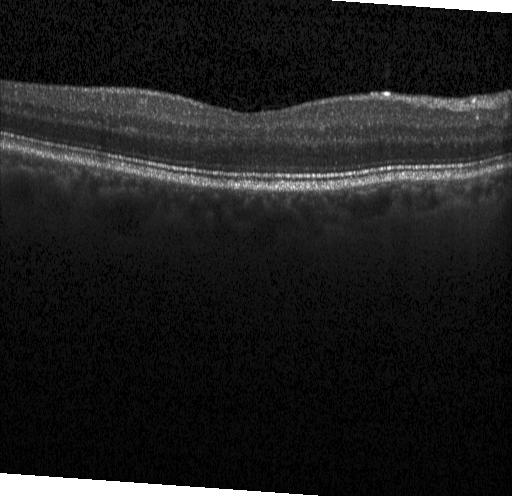 Finding: no CNV, no DME, and no drusen.